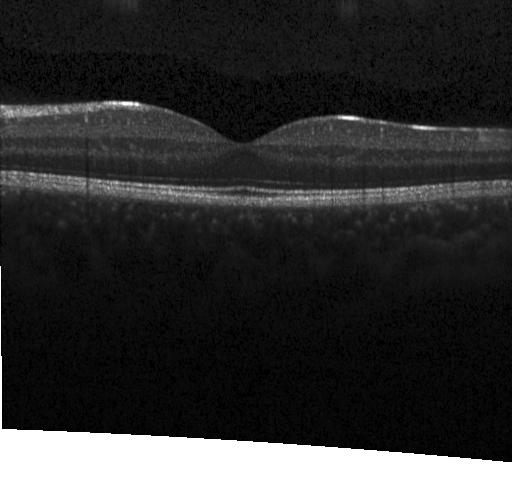

Retinal OCT cross-section — Neither CNV, DME, nor drusen.